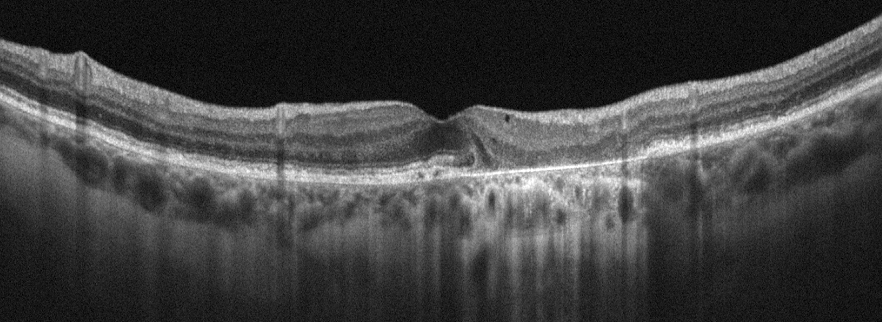

Dx: AMD.